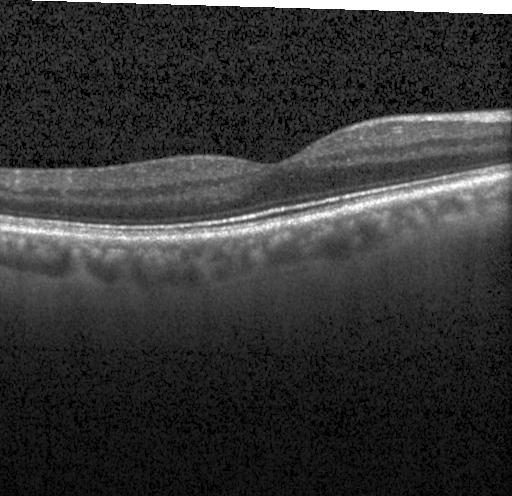

Retinal OCT cross-section; spectral-domain optical coherence tomography; fovea-centered. Assessment: no evidence of CNV, DME, or drusen.